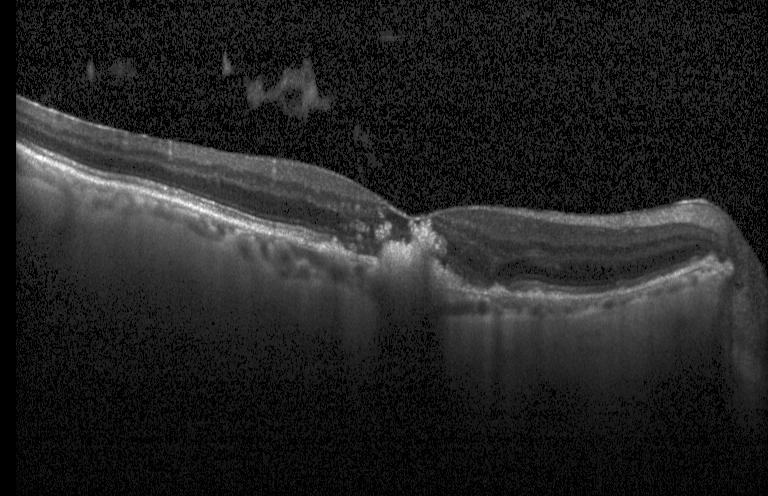
Retinal OCT cross-section. This B-scan demonstrates a choroidal neovascular membrane.